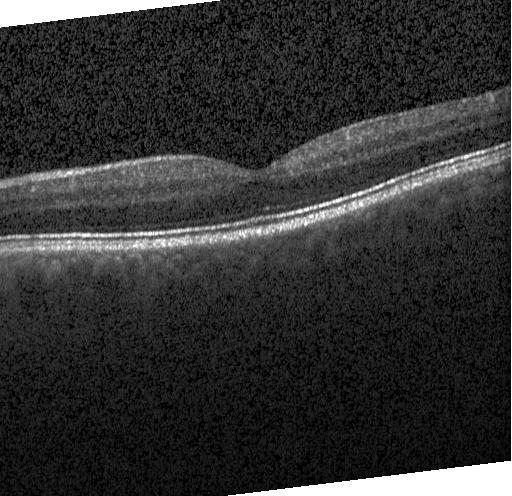
Dx: no evidence of choroidal neovascularization, diabetic macular edema, or drusen.